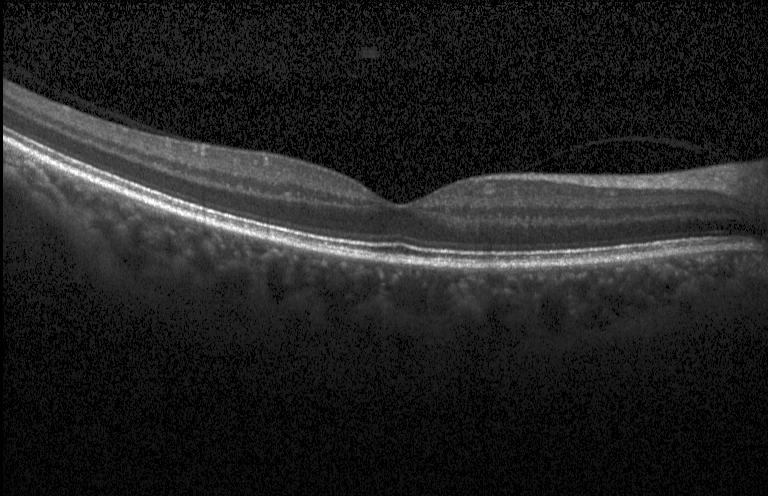 Optical coherence tomography scan. Finding: no evidence of choroidal neovascularization, diabetic macular edema, or drusen.